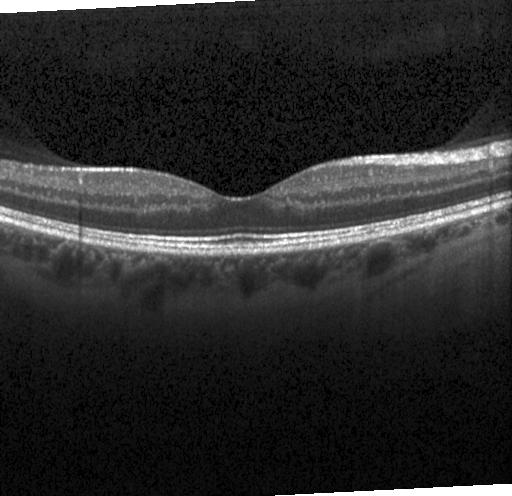 Finding: no evidence of choroidal neovascularization, diabetic macular edema, or drusen.